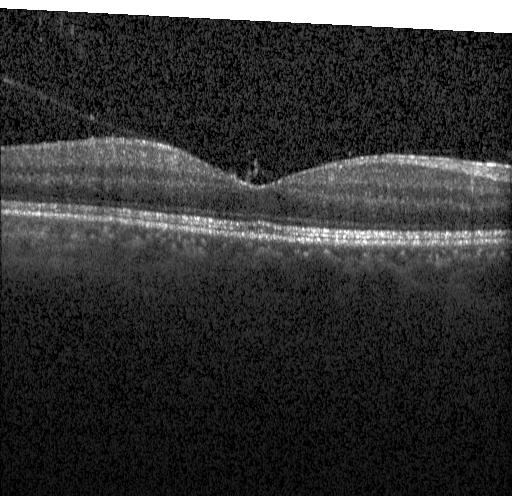
Macular OCT: no evidence of choroidal neovascularization, diabetic macular edema, or drusen.